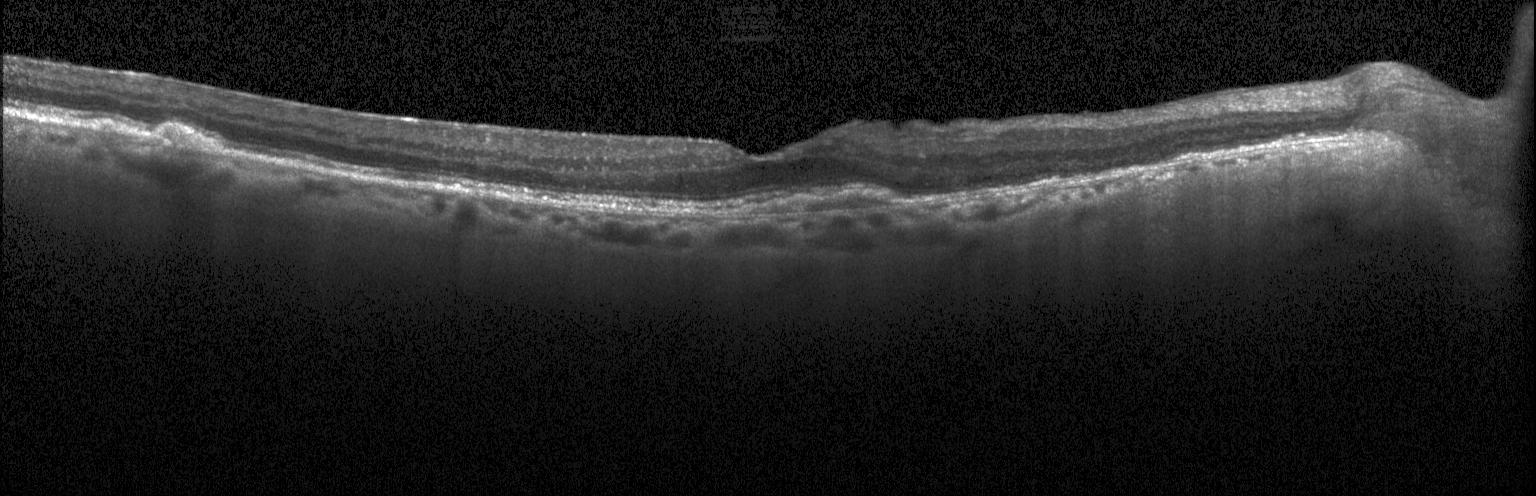

Through the macula. SD-OCT. OCT B-scan — The scan shows a choroidal neovascular membrane.